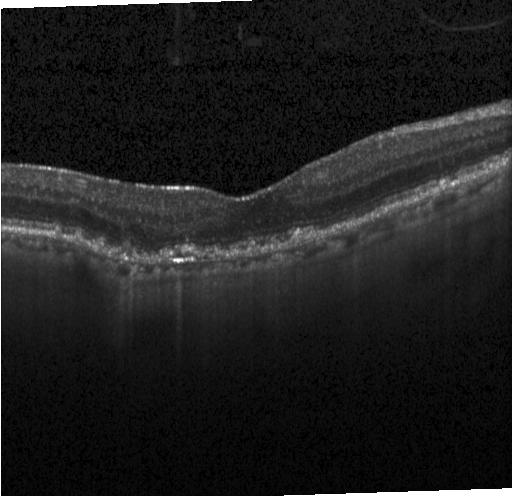
OCT scan showing a choroidal neovascular membrane.